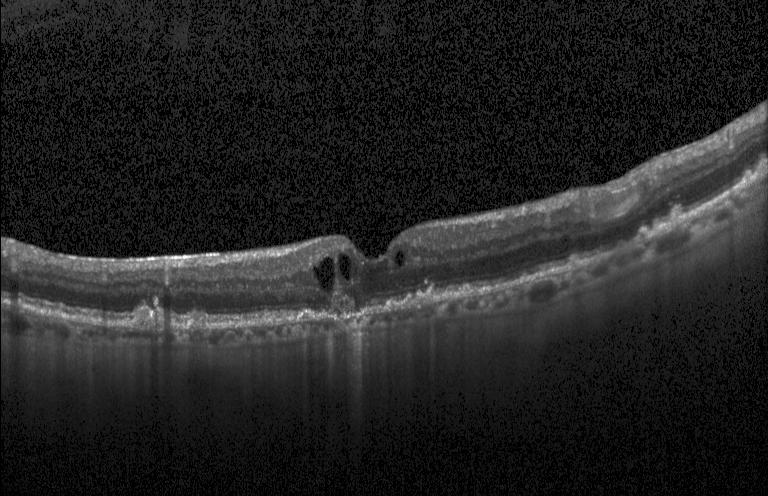

Impression: a choroidal neovascular membrane.